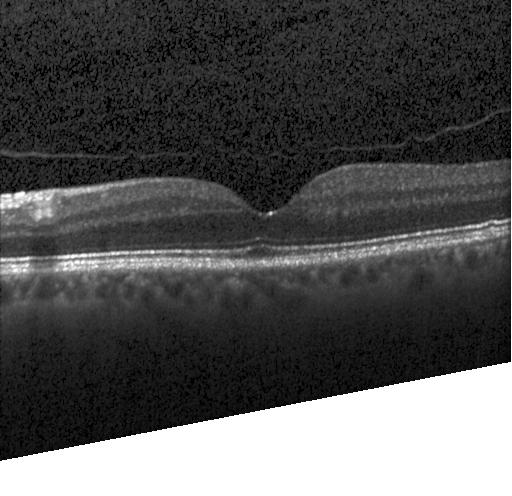 OCT B-scan. OCT finding: no choroidal neovascularization, no diabetic macular edema, and no drusen.